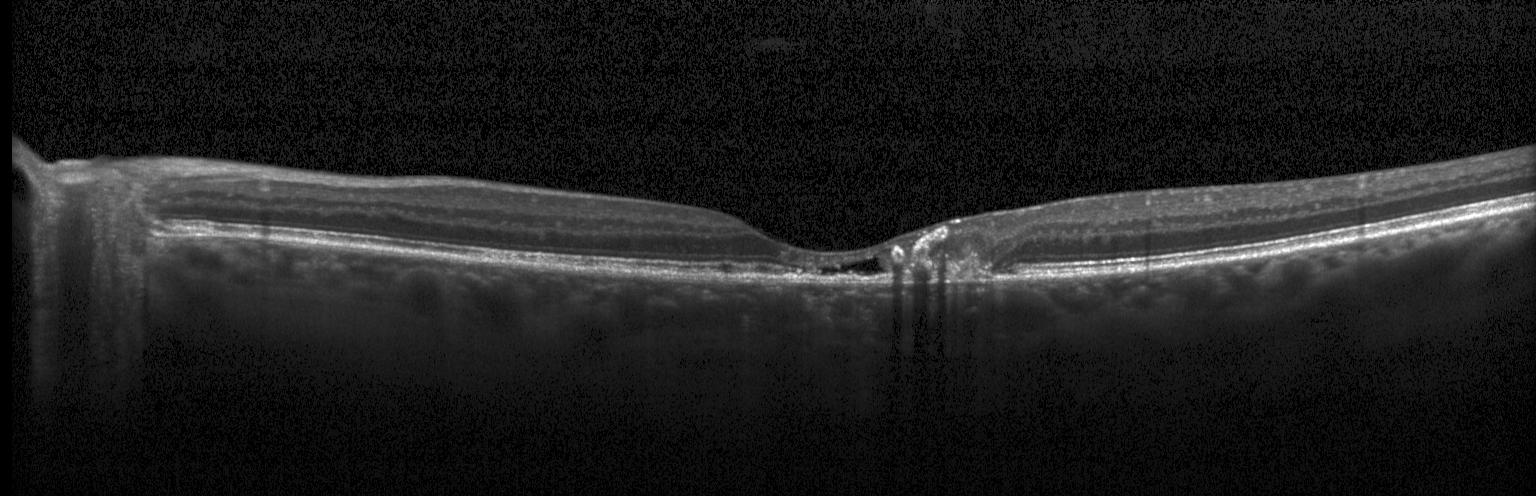

Fovea-centered; OCT line scan
Dx: a choroidal neovascular membrane.